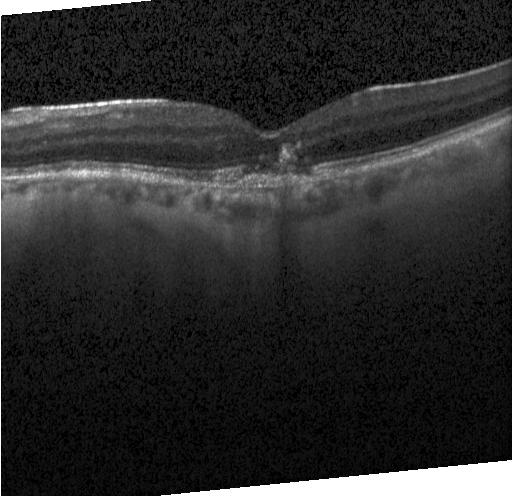

OCT line scan, spectral-domain optical coherence tomography — Impression: a choroidal neovascular membrane.